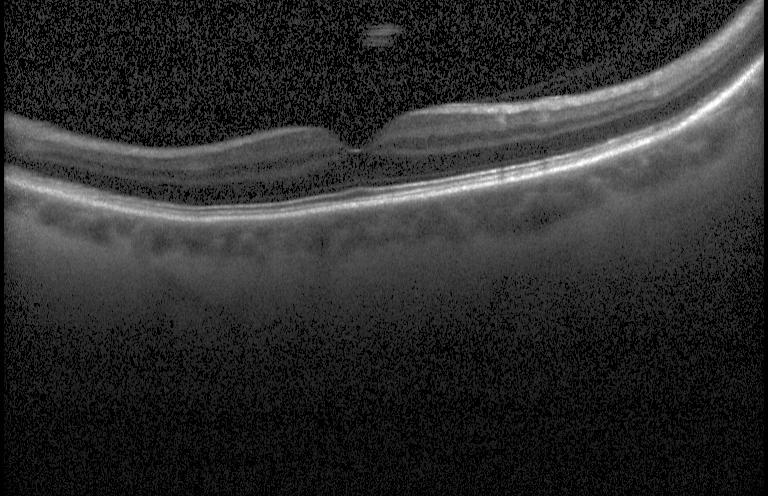

Acquired on a Heidelberg Spectralis · retinal OCT B-scan.
Impression: no choroidal neovascularization, no diabetic macular edema, and no drusen.